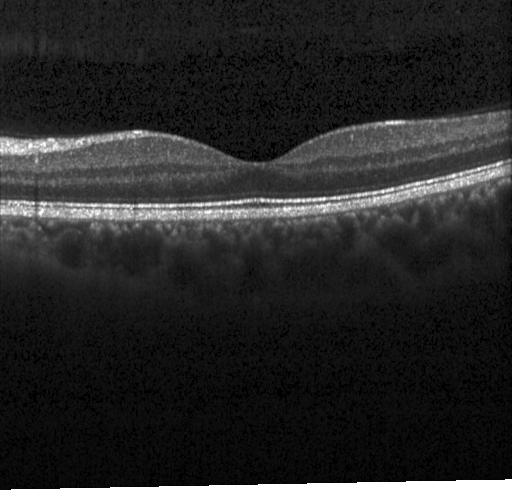

Macular OCT demonstrating no choroidal neovascularization, diabetic macular edema, or drusen.